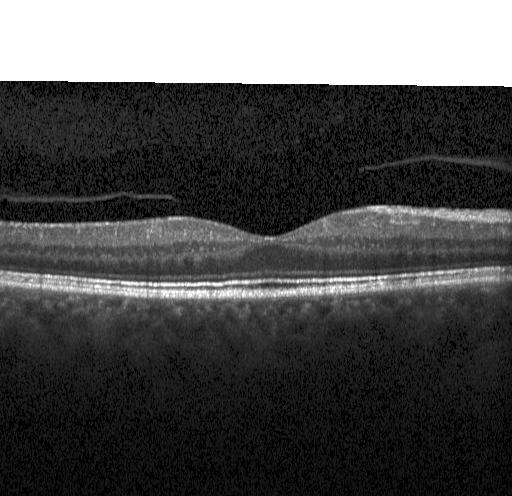
OCT B-scan · acquired on a Heidelberg Spectralis.
This B-scan demonstrates neither choroidal neovascularization, diabetic macular edema, nor drusen.